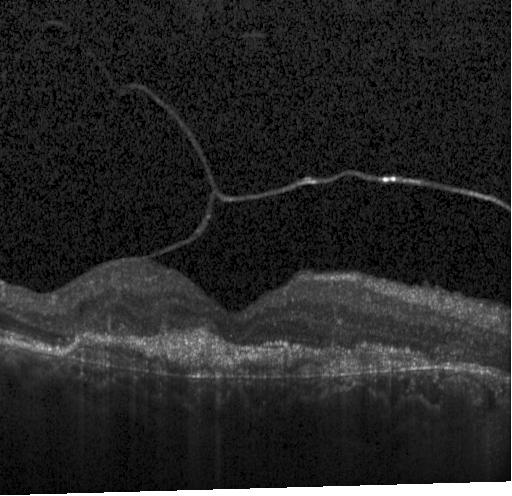
OCT line scan; through the macula — Assessment: a choroidal neovascular membrane.